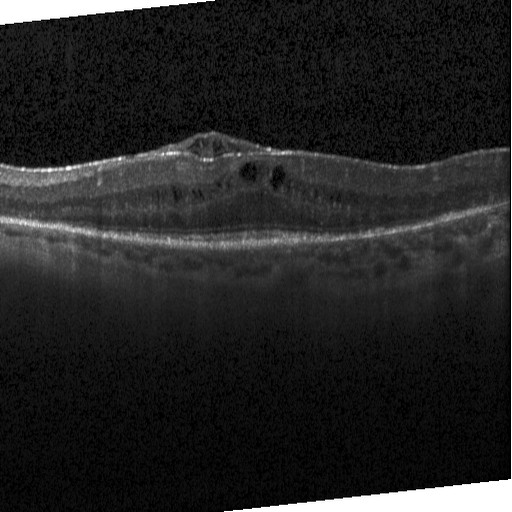 OCT B-scan.
Impression: diabetic macular edema.